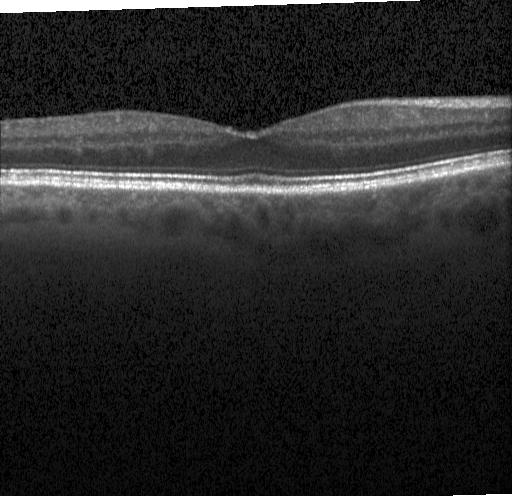 Finding: no choroidal neovascularization, diabetic macular edema, or drusen.